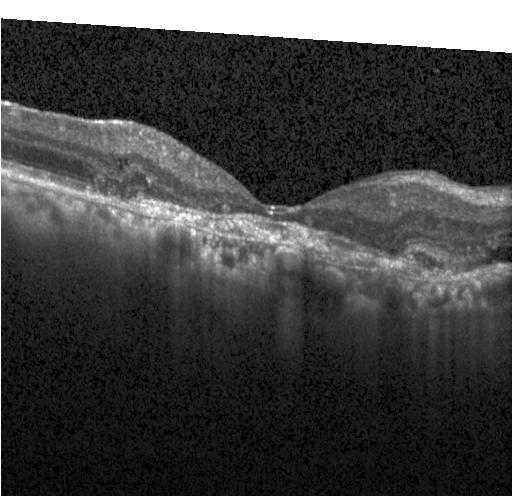

Retinal OCT cross-section showing a choroidal neovascular membrane.